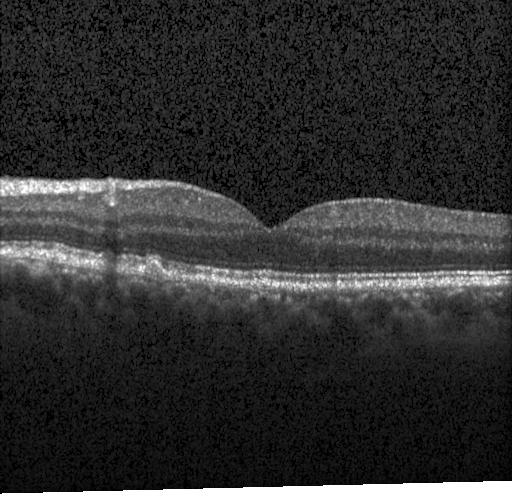 Multiple drusen.